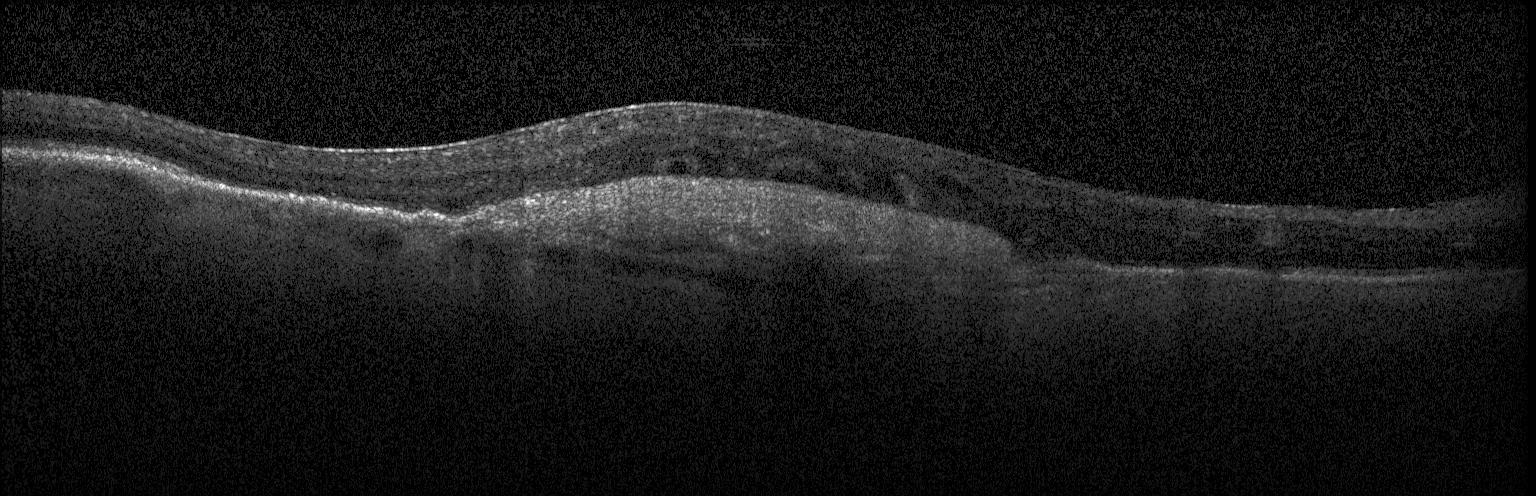
SD-OCT · OCT B-scan
Choroidal neovascularization (CNV).